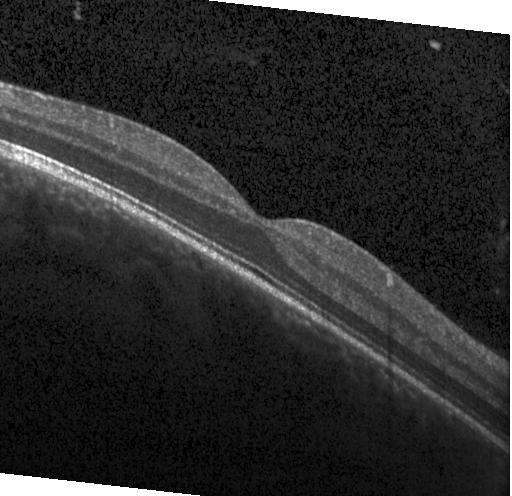

Assessment: neither choroidal neovascularization, diabetic macular edema, nor drusen.